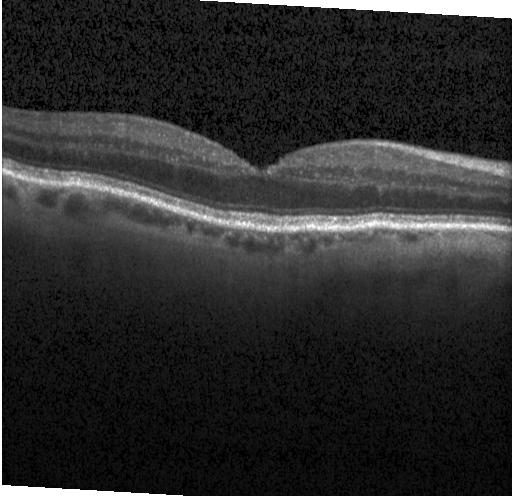

Finding: neither choroidal neovascularization, diabetic macular edema, nor drusen.